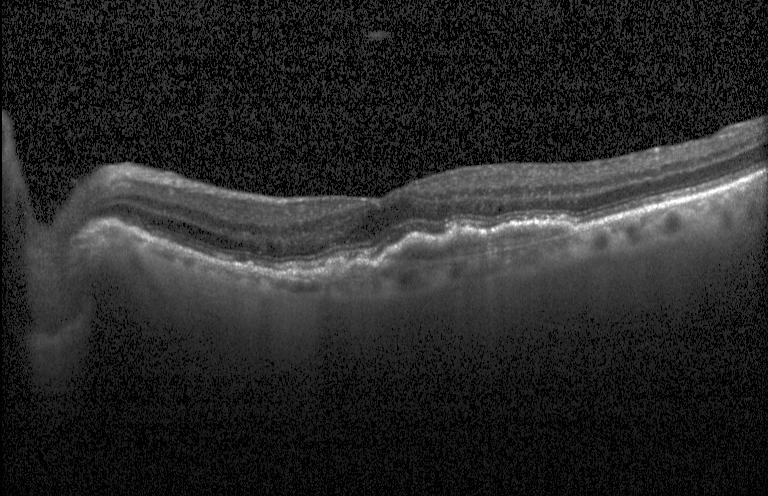 SD-OCT; through the macula; Heidelberg Spectralis; optical coherence tomography B-scan.
Macular OCT: choroidal neovascularization.